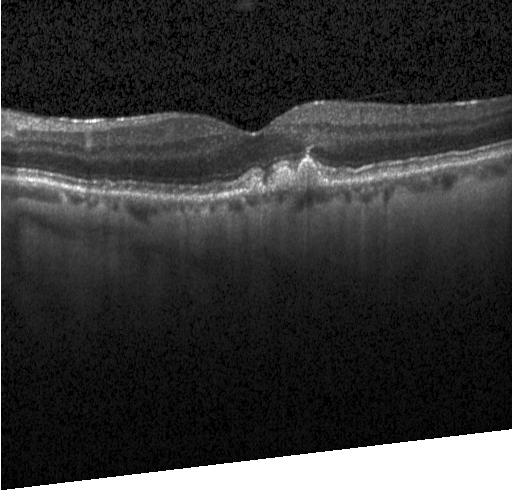 Retinal OCT B-scan.
Diagnosis: drusen.